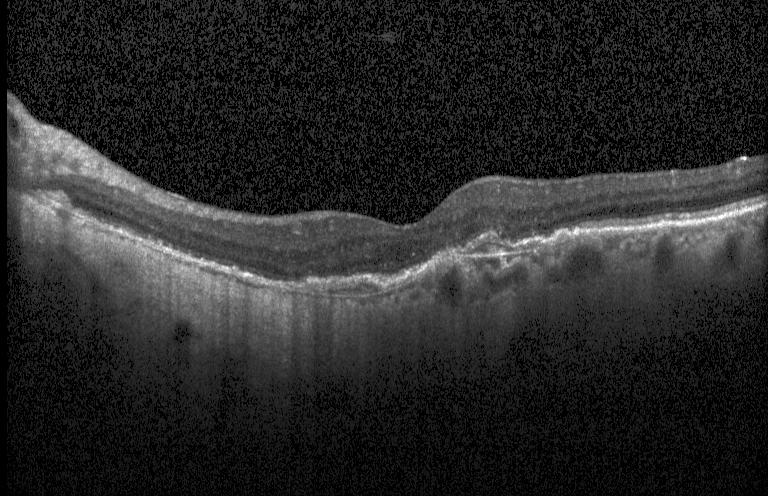 Macular OCT demonstrating a choroidal neovascular membrane.